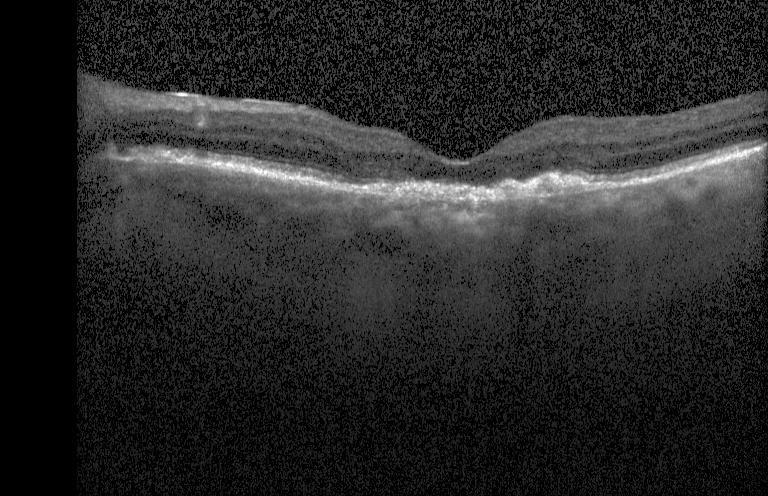 Spectral-domain optical coherence tomography · optical coherence tomography B-scan · Heidelberg Spectralis.
A choroidal neovascular membrane.